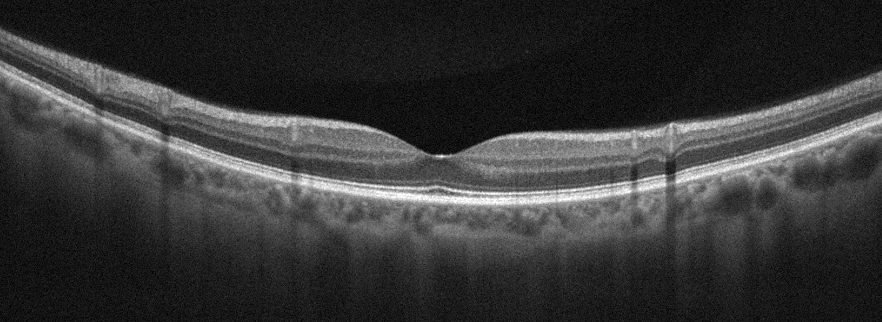 Impression: no AMD, DME, ERM, RAO, RVO, or VID.